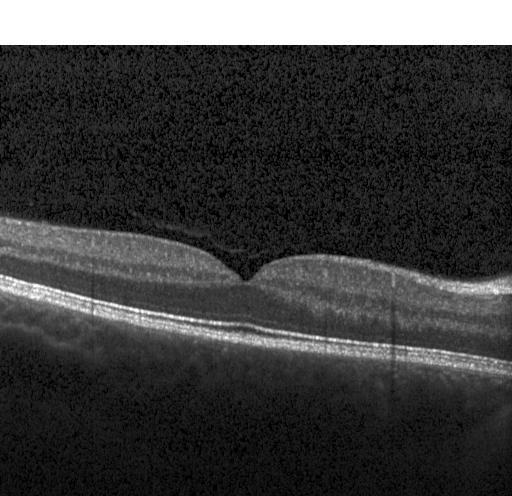

Finding: no CNV, DME, or drusen.